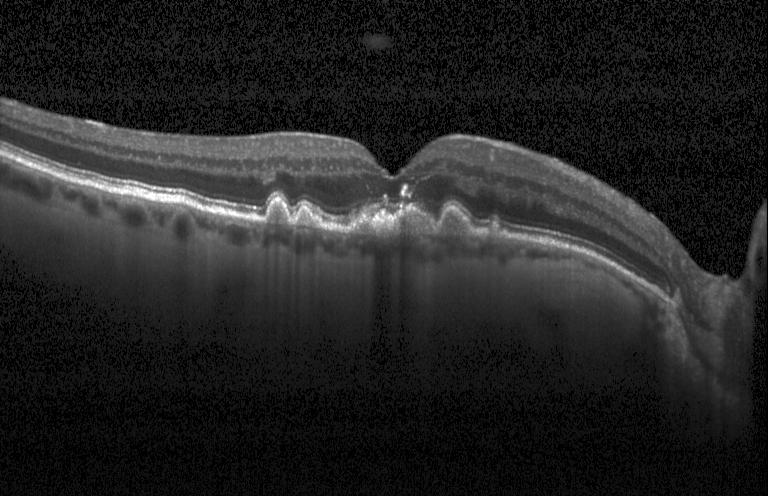 Retinal OCT B-scan · fovea-centered · acquired on a Heidelberg Spectralis
Finding: sub-RPE drusenoid deposits.